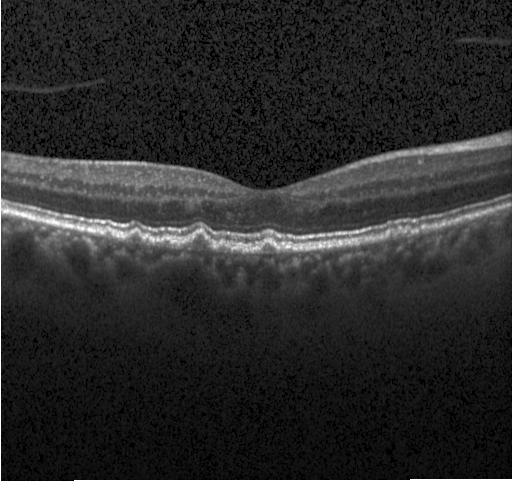
The scan shows sub-RPE drusenoid deposits.